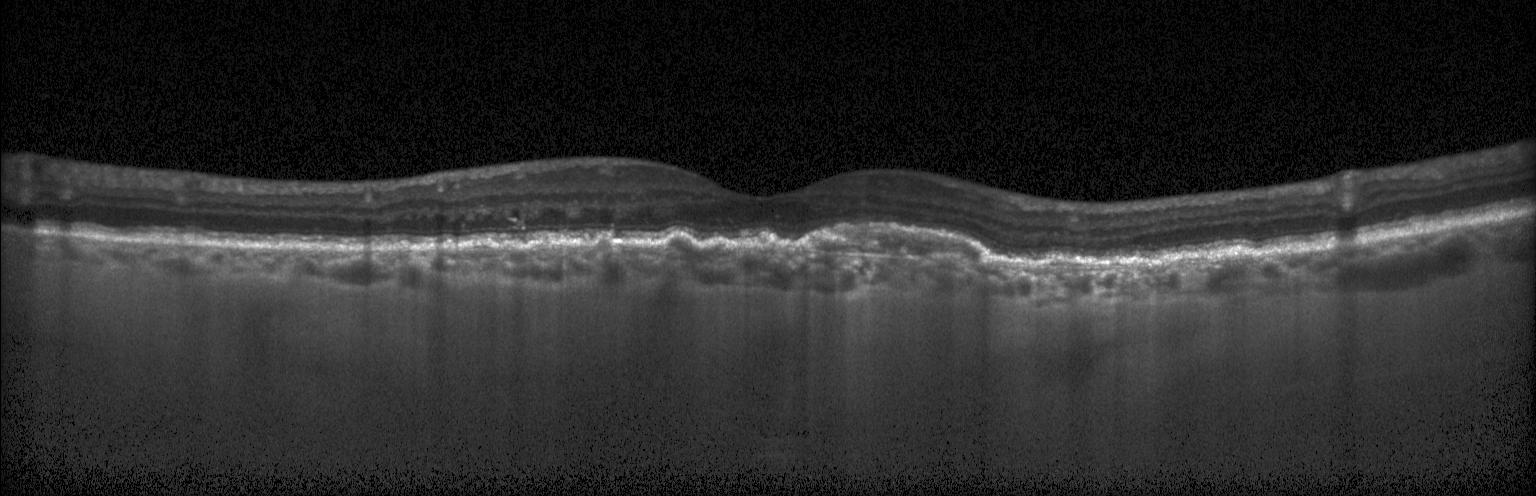

Optical coherence tomography B-scan, SD-OCT. CNV.